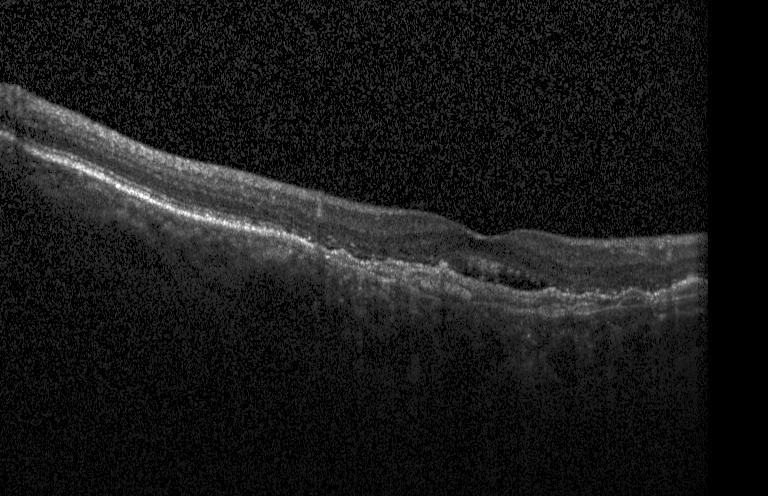 OCT line scan
The scan shows CNV.